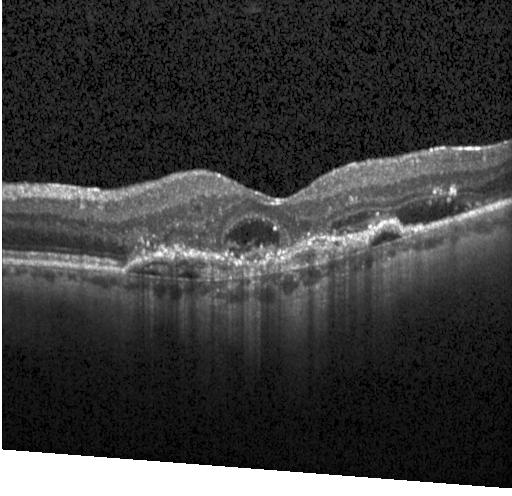

Spectral-domain optical coherence tomography. Retinal OCT cross-section. Acquired on a Heidelberg Spectralis. Diagnosis: a choroidal neovascular membrane.